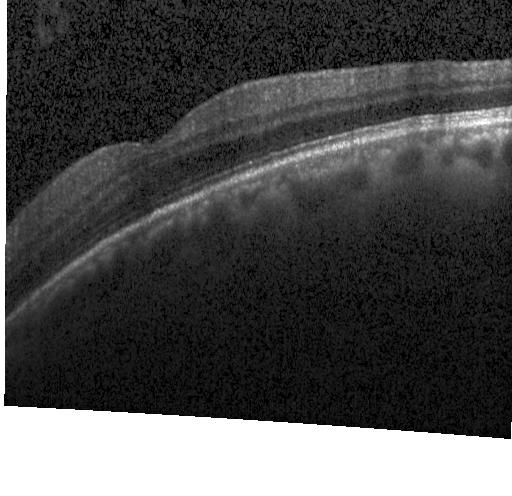
OCT B-scan showing no choroidal neovascularization, no diabetic macular edema, and no drusen.